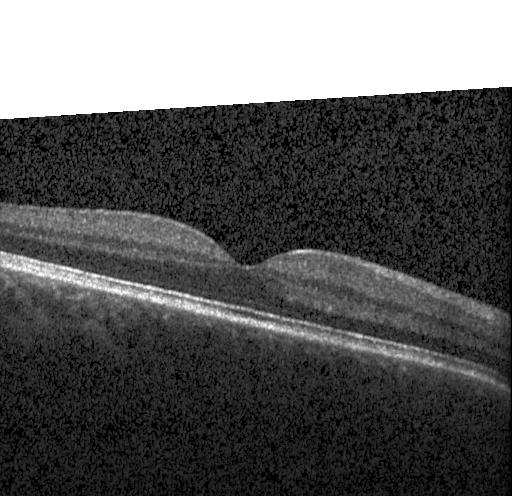
Assessment: neither choroidal neovascularization, diabetic macular edema, nor drusen.